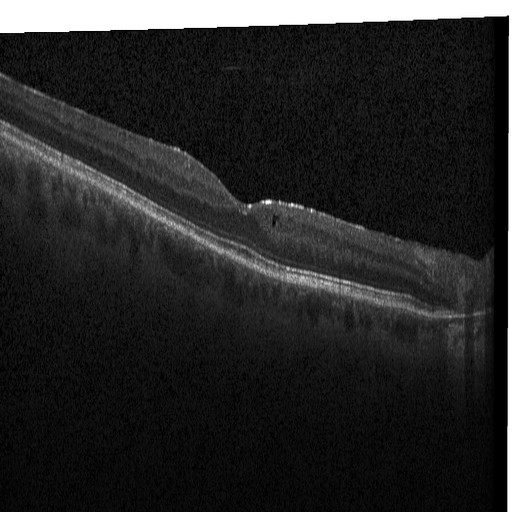
OCT scan showing diabetic macular edema (DME).